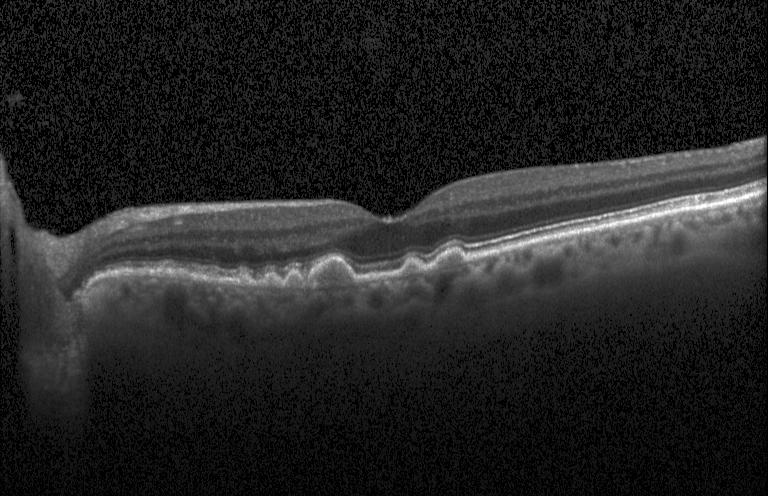

OCT B-scan.
Finding: sub-RPE drusenoid deposits.